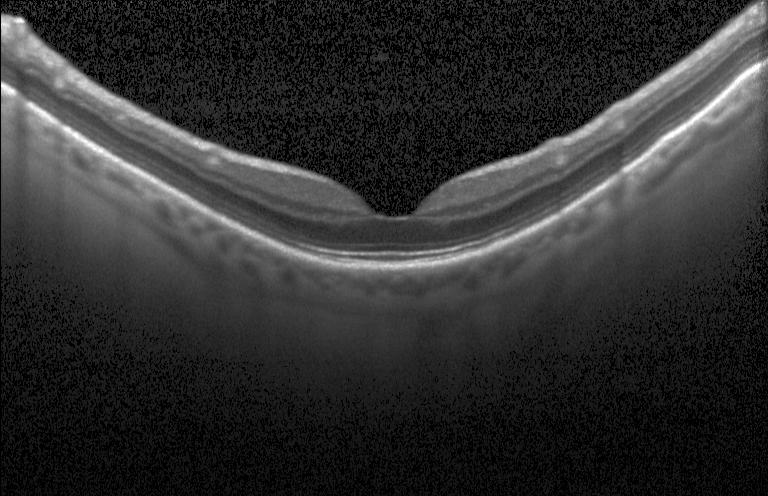
Instrument: Heidelberg Spectralis, SD-OCT, horizontal scan through the fovea, OCT line scan
Impression: no CNV, DME, or drusen.